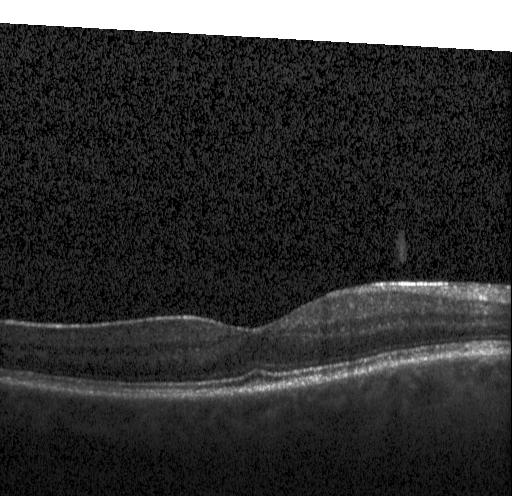

Finding: no evidence of CNV, DME, or drusen.